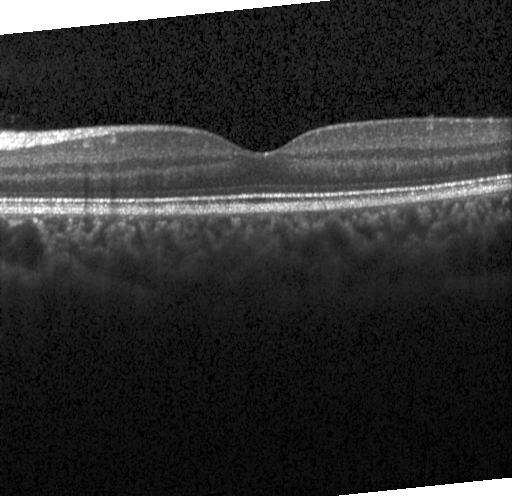
Diagnosis: neither CNV, DME, nor drusen.